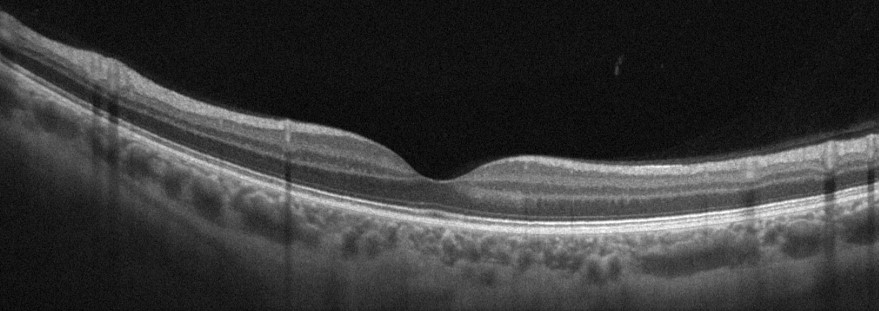 Retinal OCT B-scan · instrument: Optovue Avanti RTVue XR — Finding: no AMD, DME, ERM, RAO, RVO, or VID.